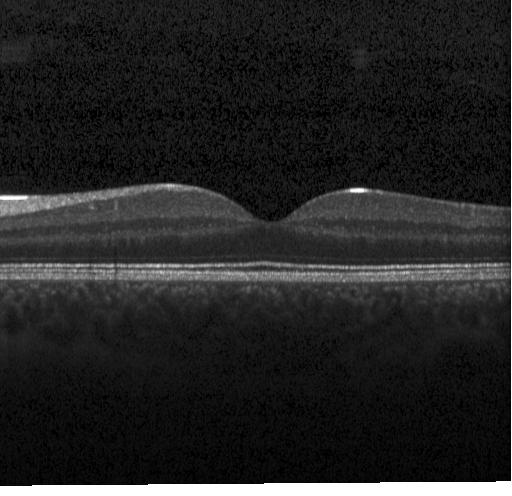

Impression: no CNV, no DME, and no drusen.